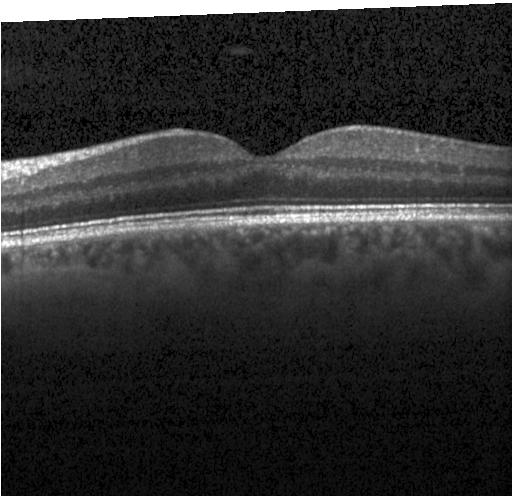 Finding: no evidence of choroidal neovascularization, diabetic macular edema, or drusen.